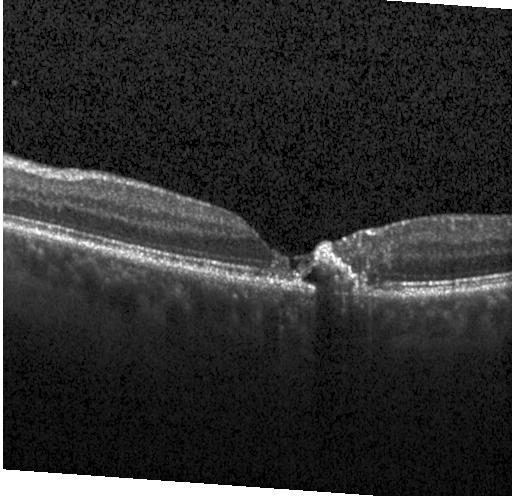 This B-scan demonstrates choroidal neovascularization (CNV).